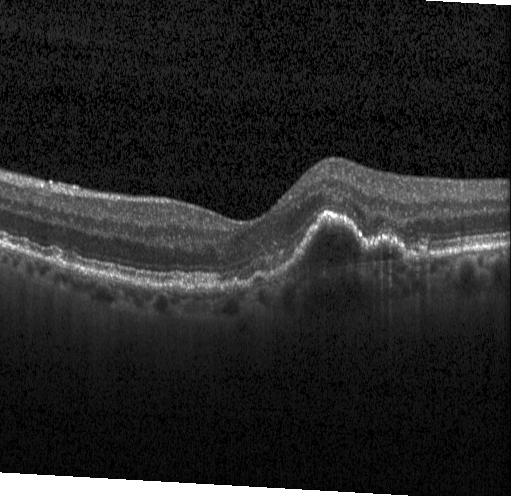

Horizontal scan through the fovea · retinal OCT B-scan · spectral-domain optical coherence tomography · acquired on a Heidelberg Spectralis. The scan shows a choroidal neovascular membrane.